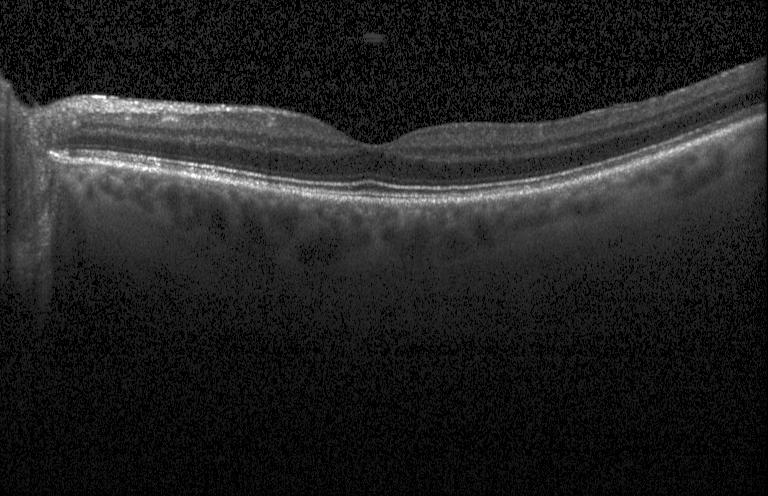
Retinal OCT B-scan.
Diagnosis: no choroidal neovascularization, diabetic macular edema, or drusen.